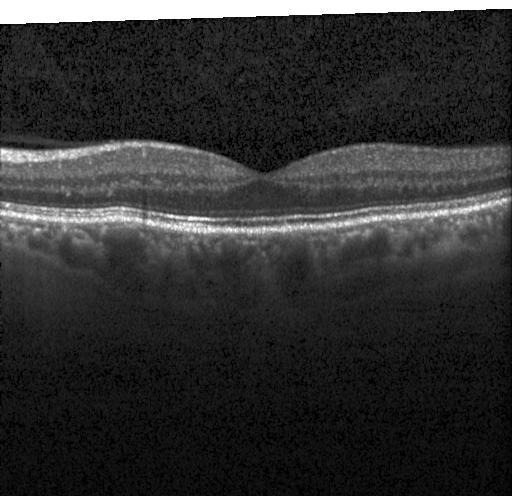
Retinal OCT B-scan.
This B-scan demonstrates neither choroidal neovascularization, diabetic macular edema, nor drusen.